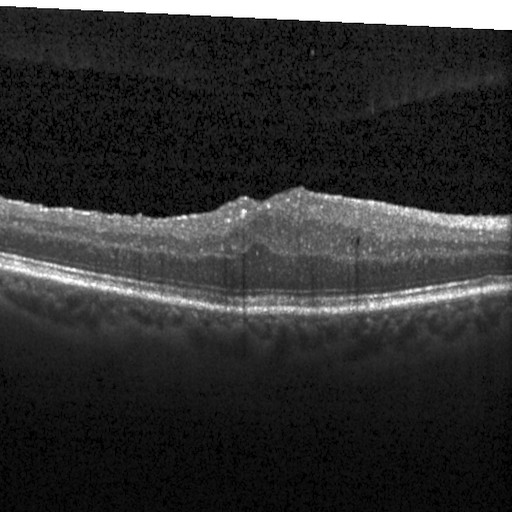

SD-OCT, fovea-centered, optical coherence tomography B-scan — Finding: diabetic macular edema.